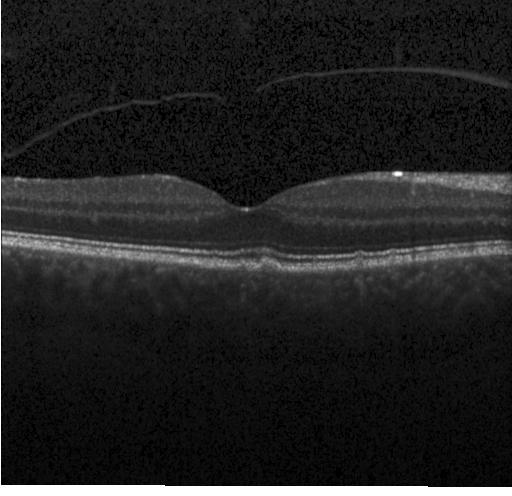
Optical coherence tomography B-scan; Heidelberg Spectralis OCT system — The scan shows sub-RPE drusenoid deposits.